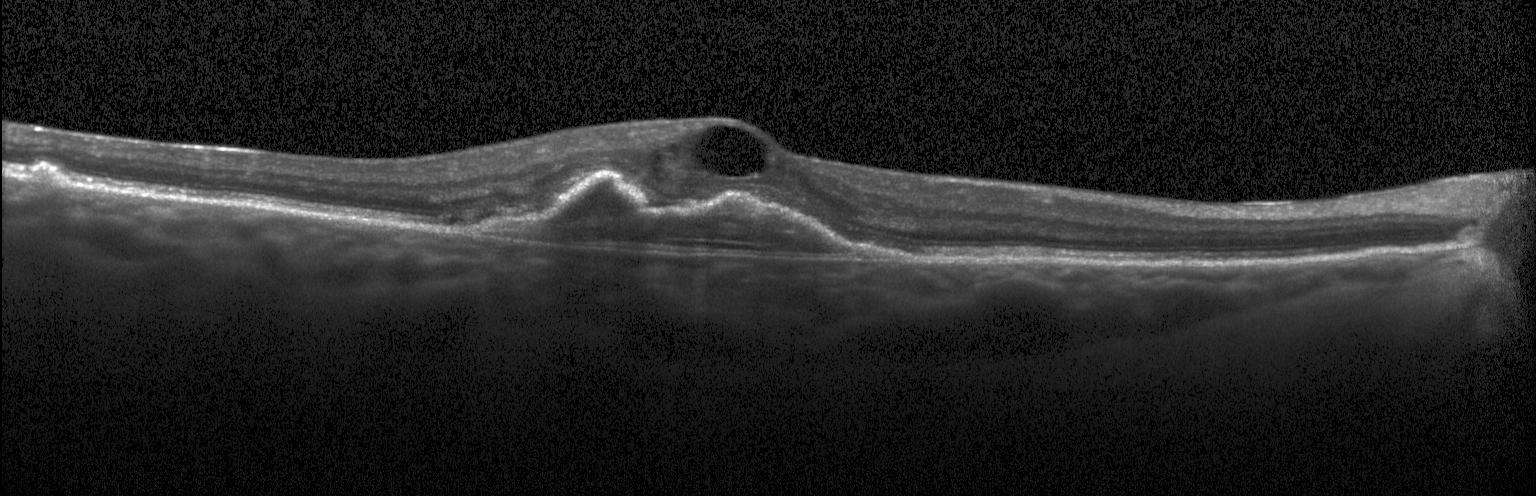 Finding: choroidal neovascularization.